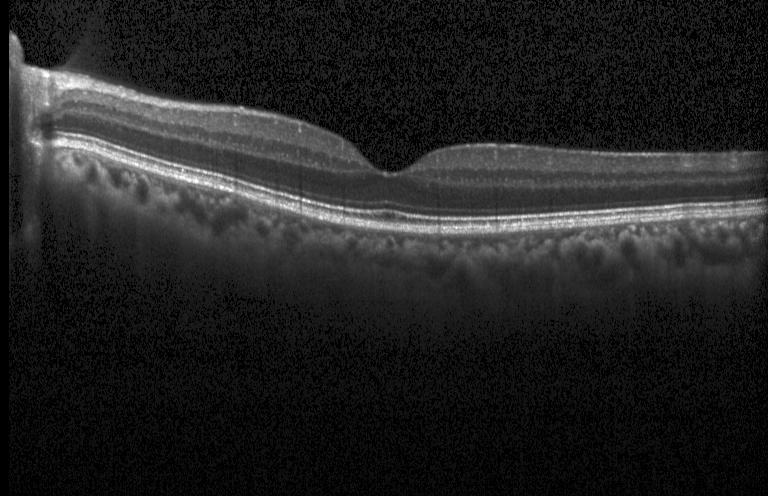
Finding: no choroidal neovascularization, no diabetic macular edema, and no drusen.